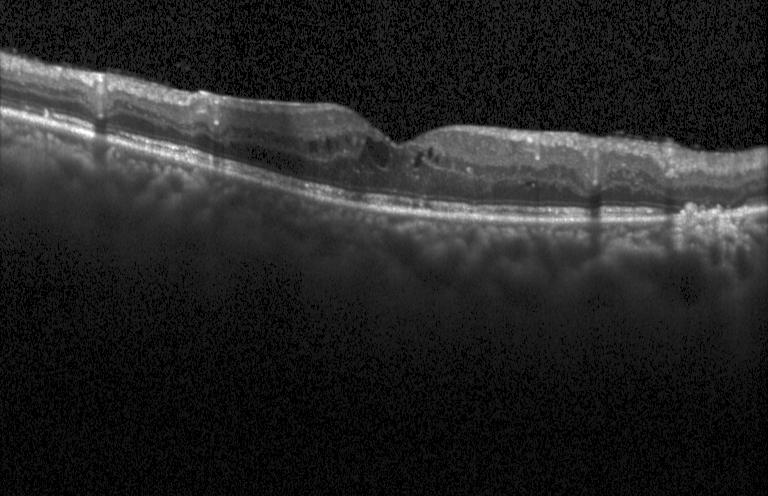
Impression: DME.